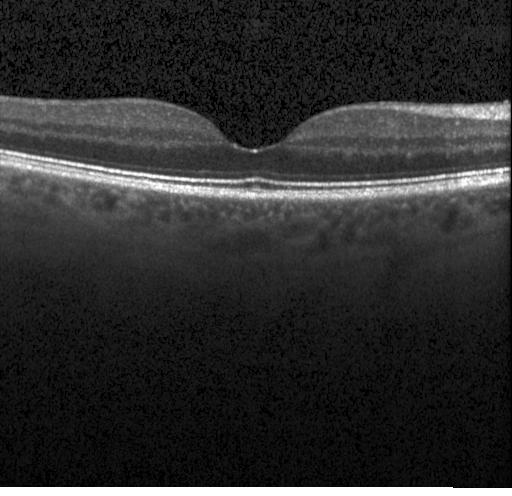
Spectral-domain OCT; retinal OCT cross-section; centered on the fovea
Macular OCT: no evidence of choroidal neovascularization, diabetic macular edema, or drusen.